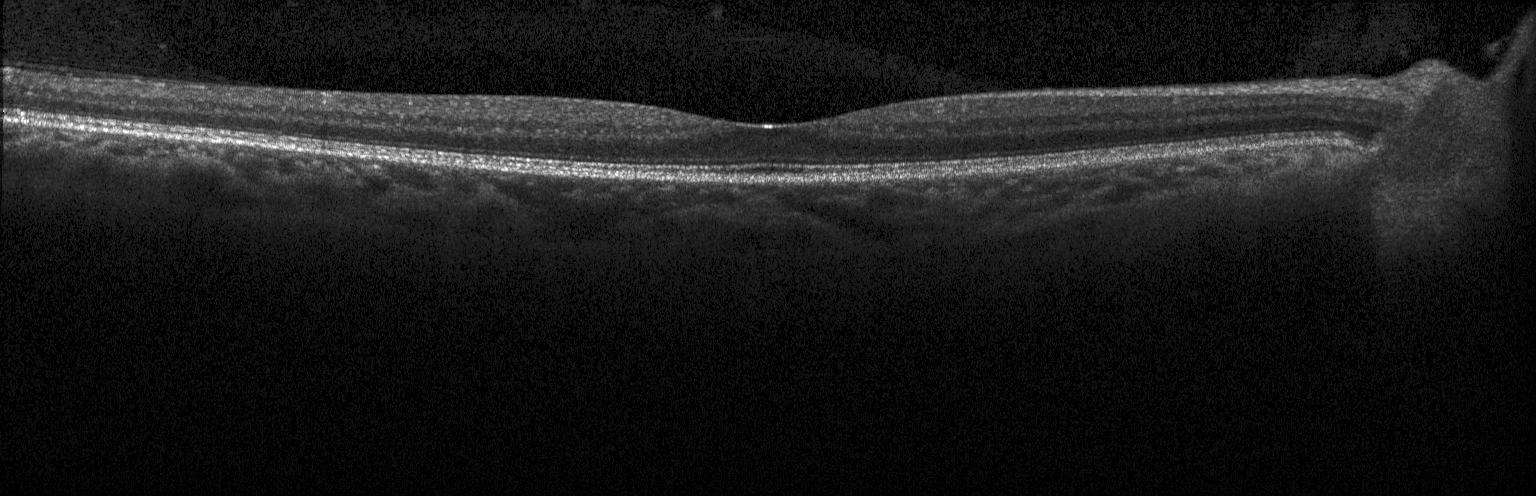 Optical coherence tomography B-scan; acquired on a Heidelberg Spectralis. Finding: no evidence of CNV, DME, or drusen.